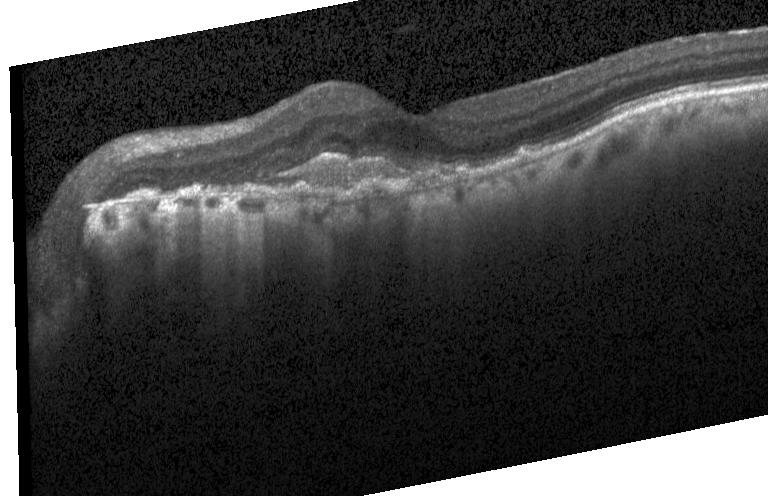
Impression: choroidal neovascularization (CNV).